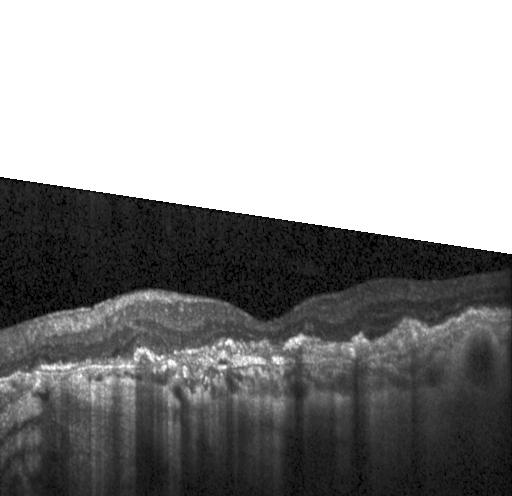

Spectral-domain optical coherence tomography, fovea-centered, retinal OCT B-scan.
Macular OCT: choroidal neovascularization.